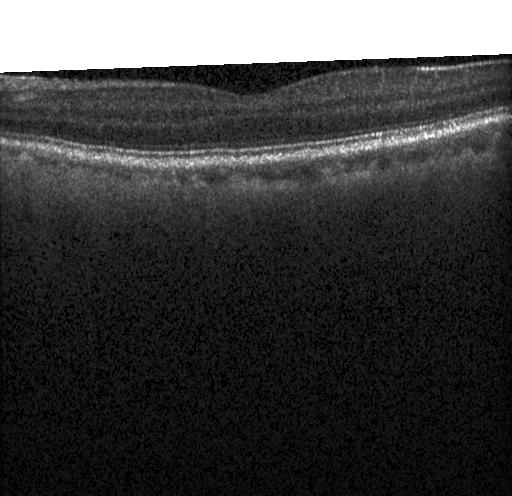 OCT line scan
The scan shows no choroidal neovascularization, diabetic macular edema, or drusen.